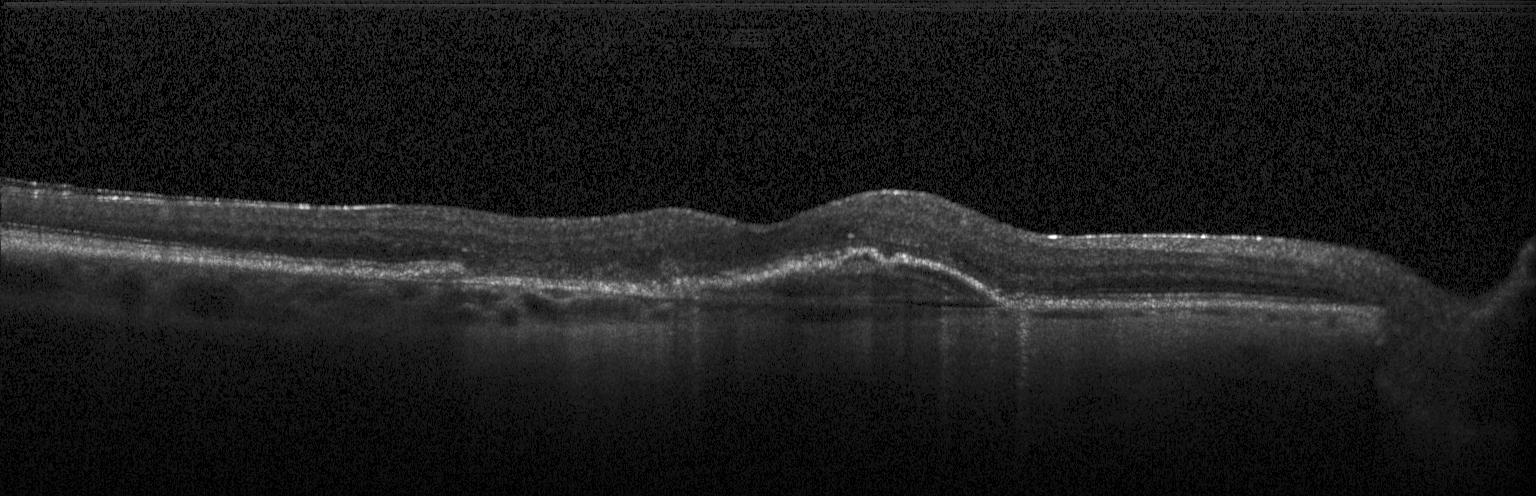
Heidelberg Spectralis OCT system, spectral-domain optical coherence tomography, horizontal scan through the fovea, OCT B-scan — This B-scan demonstrates choroidal neovascularization (CNV).